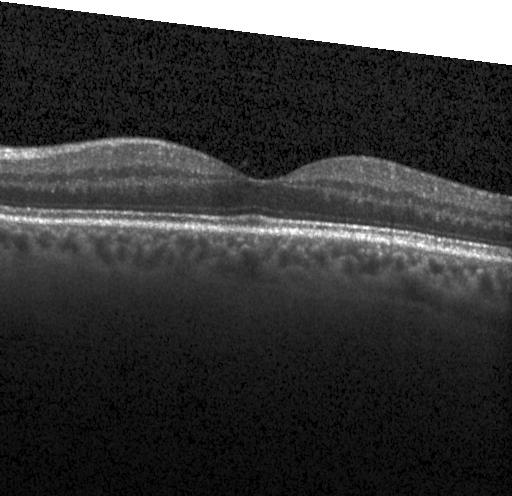 SD-OCT; through the macula; Heidelberg Spectralis; optical coherence tomography B-scan
Neither CNV, DME, nor drusen.